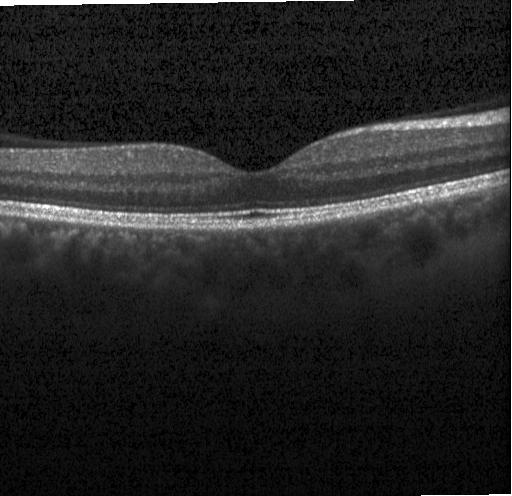

Heidelberg Spectralis; horizontal scan through the fovea; spectral-domain OCT; retinal OCT cross-section
Finding: neither choroidal neovascularization, diabetic macular edema, nor drusen.